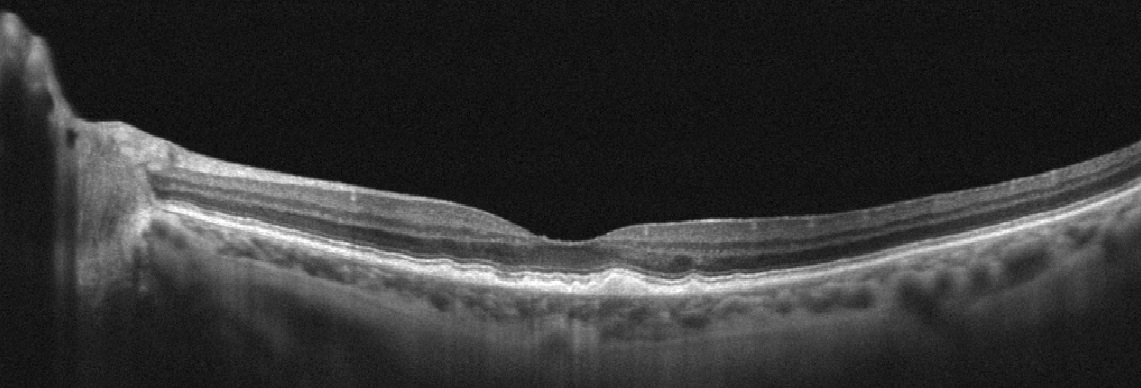

Retinal OCT cross-section showing age-related macular degeneration.